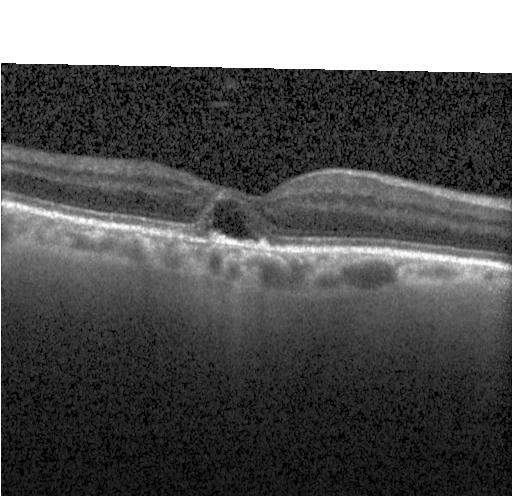
Dx: a choroidal neovascular membrane.